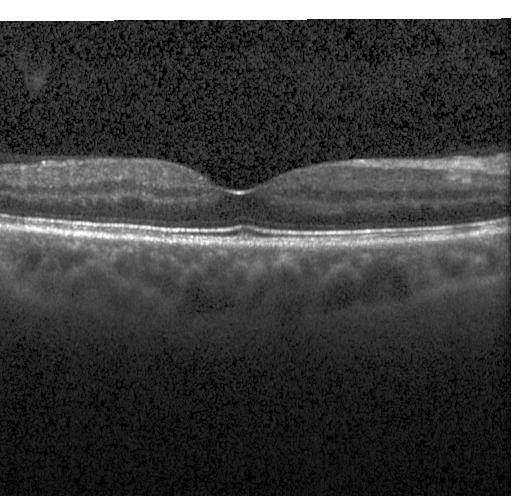
OCT line scan · fovea-centered. Impression: no evidence of choroidal neovascularization, diabetic macular edema, or drusen.